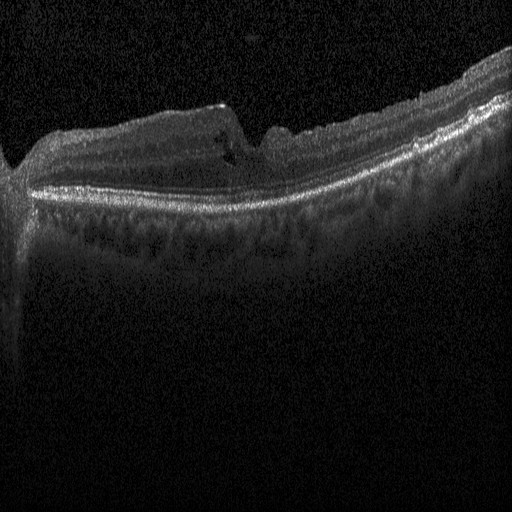 Macular OCT: DME.